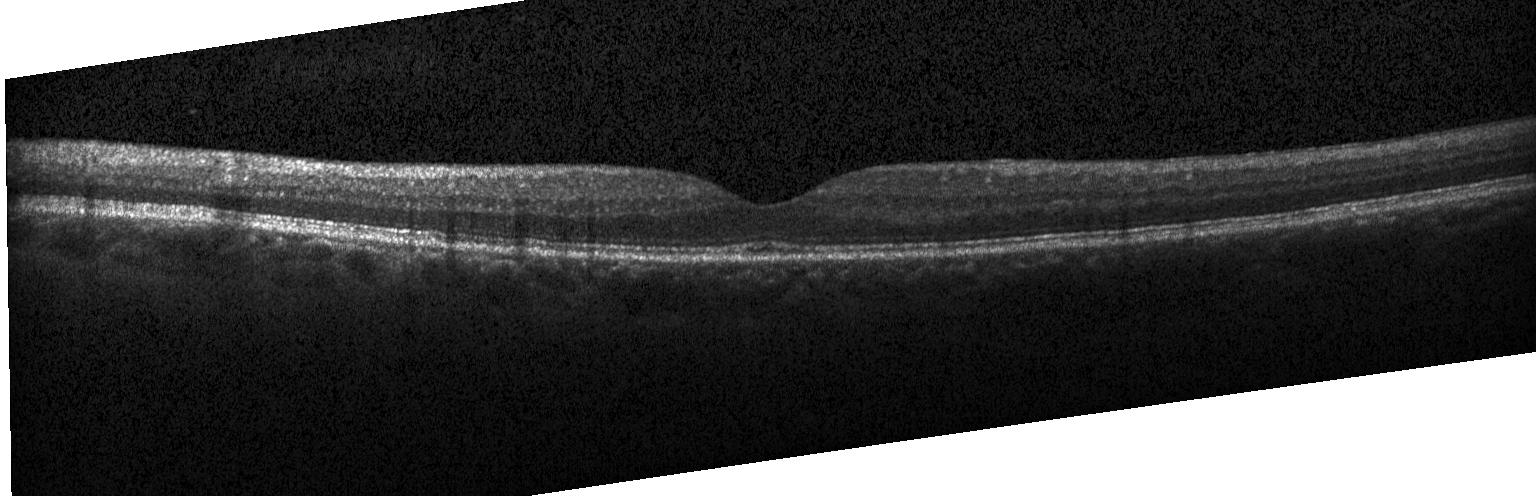 Through the macula. Retinal OCT cross-section. This B-scan demonstrates no CNV, no DME, and no drusen.